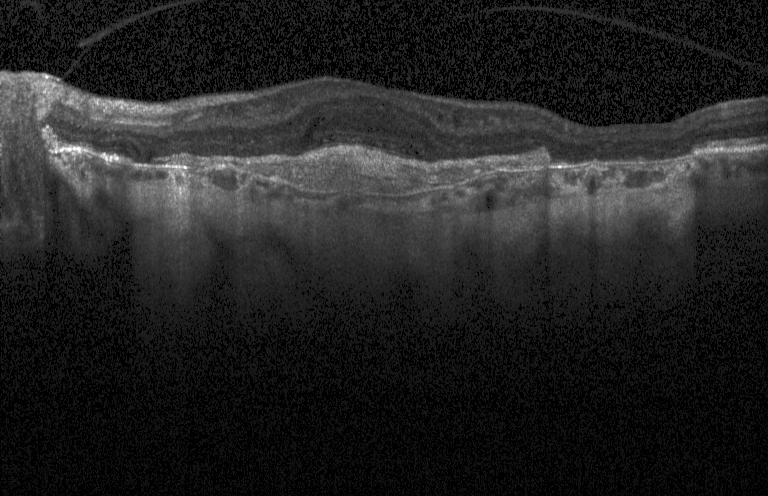 The scan shows a choroidal neovascular membrane.